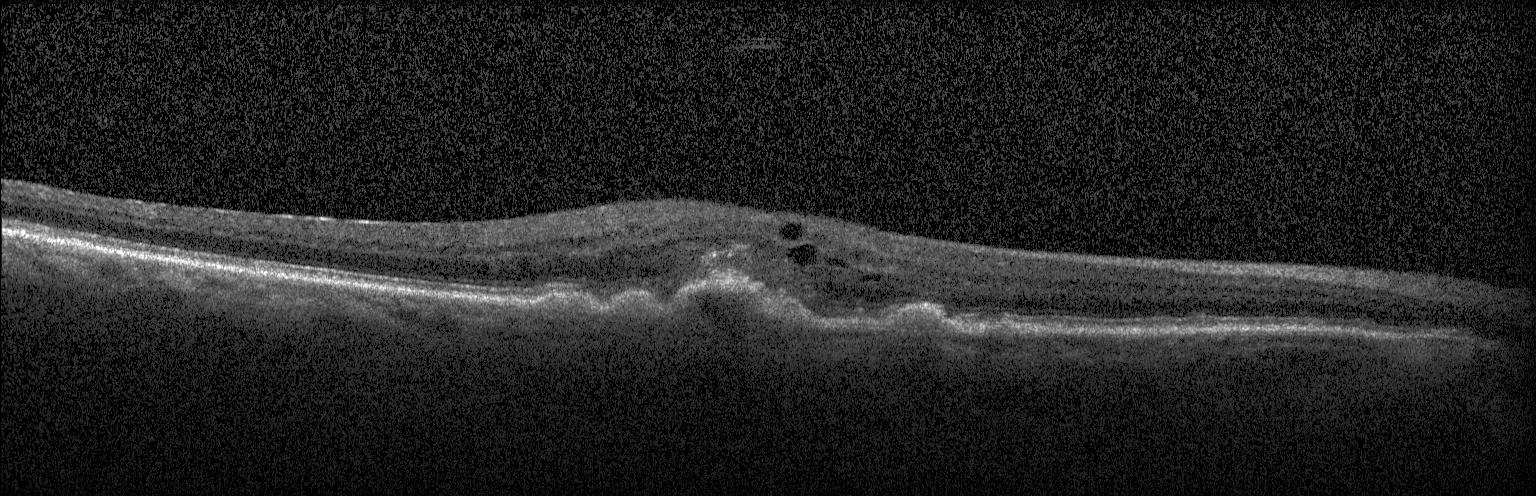
This B-scan demonstrates a choroidal neovascular membrane.